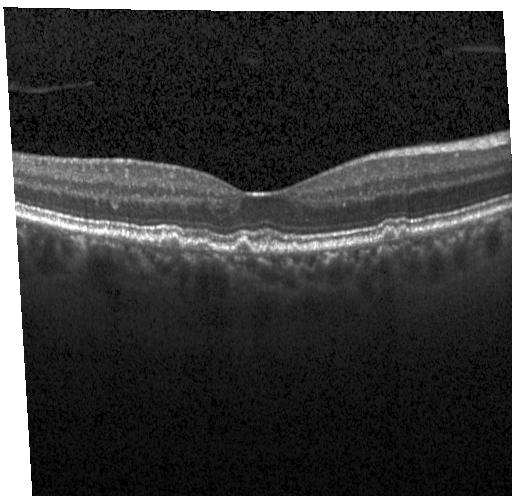
Retinal OCT cross-section showing drusen.